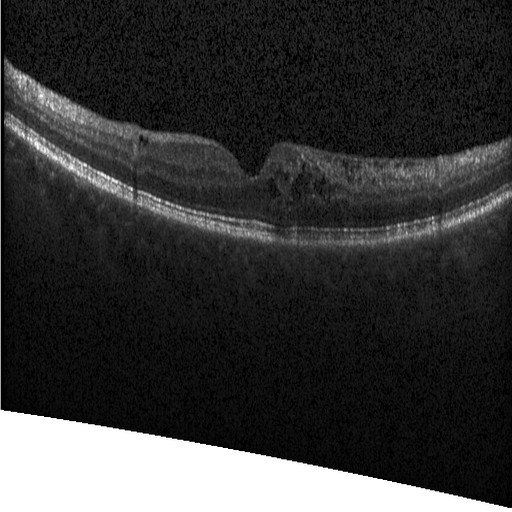

Macular OCT: DME.